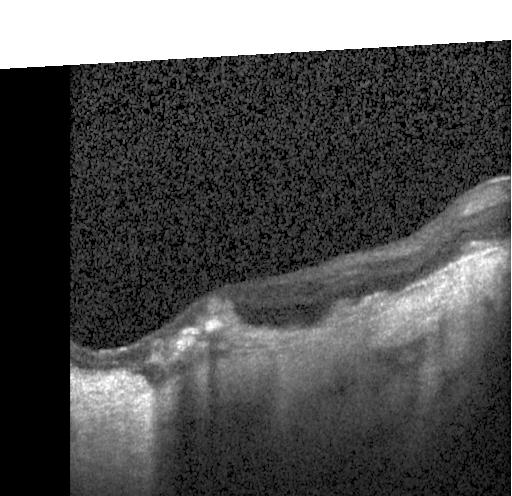
Retinal OCT cross-section, spectral-domain optical coherence tomography — This B-scan demonstrates choroidal neovascularization (CNV).